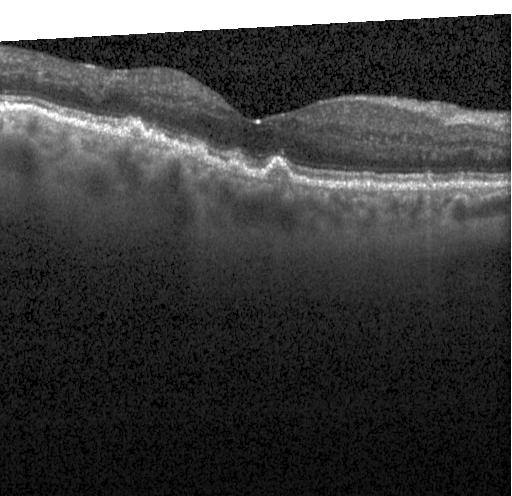

Centered on the fovea, spectral-domain OCT, Heidelberg Spectralis, OCT B-scan. OCT finding: sub-RPE drusenoid deposits.